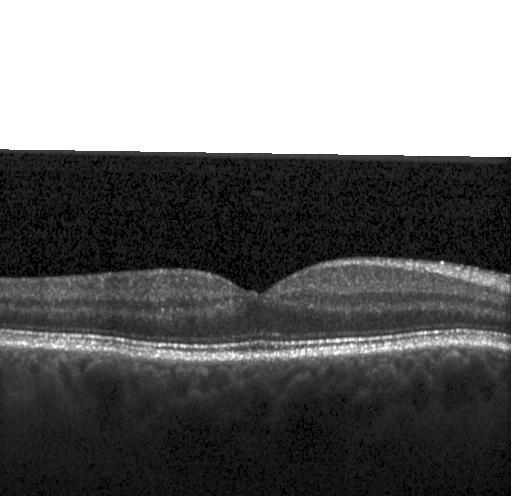
OCT B-scan, spectral-domain optical coherence tomography, through the macula, instrument: Heidelberg Spectralis.
No evidence of choroidal neovascularization, diabetic macular edema, or drusen.